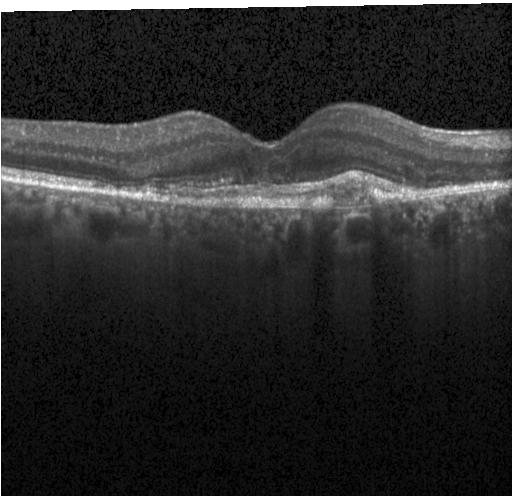 Macular OCT: CNV.